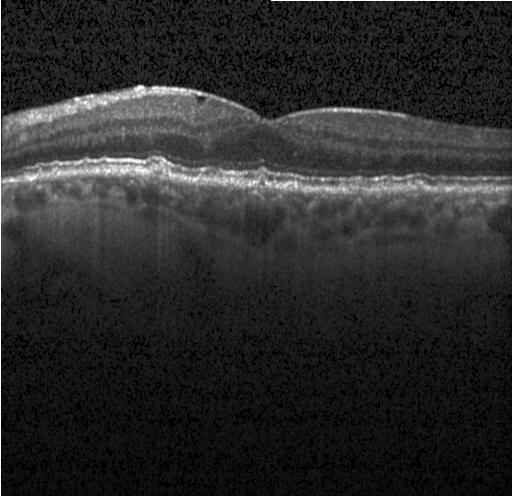

OCT line scan
Assessment: sub-RPE drusenoid deposits.